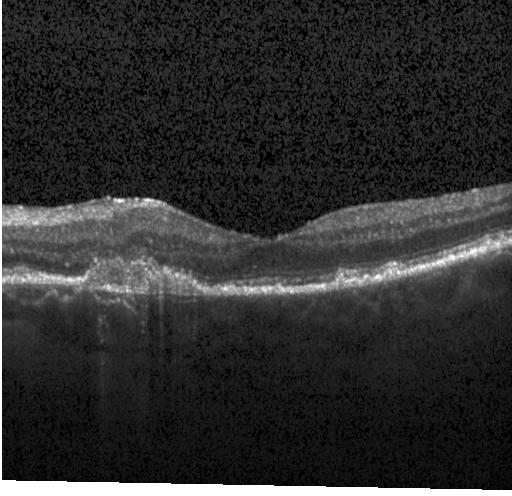
Spectral-domain optical coherence tomography; centered on the fovea; Heidelberg Spectralis; retinal OCT cross-section
This B-scan demonstrates choroidal neovascularization.